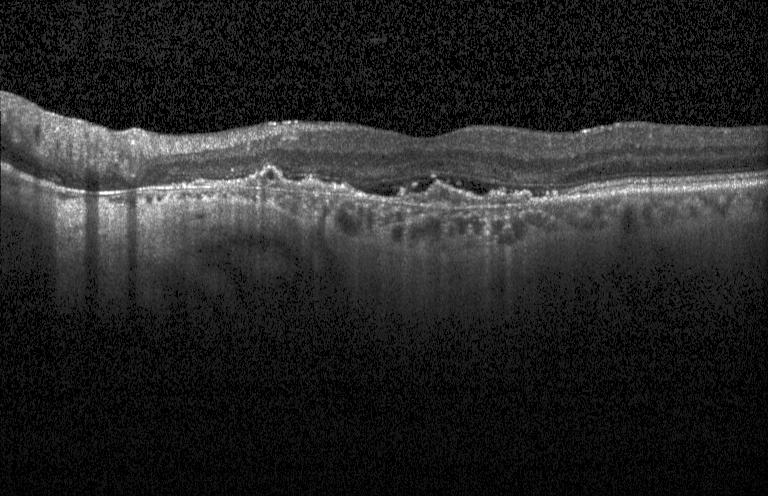

Retinal OCT cross-section.
OCT finding: choroidal neovascularization.